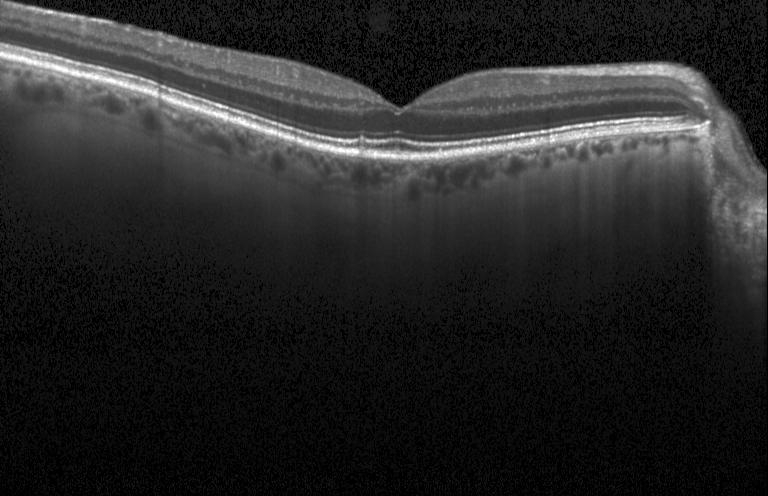 Macular OCT demonstrating neither CNV, DME, nor drusen.